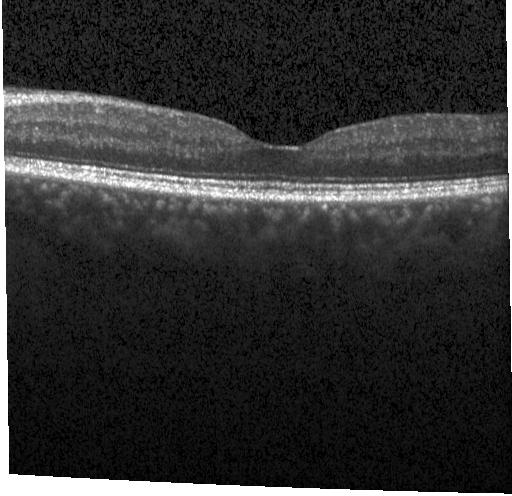

Macular OCT demonstrating no CNV, DME, or drusen.